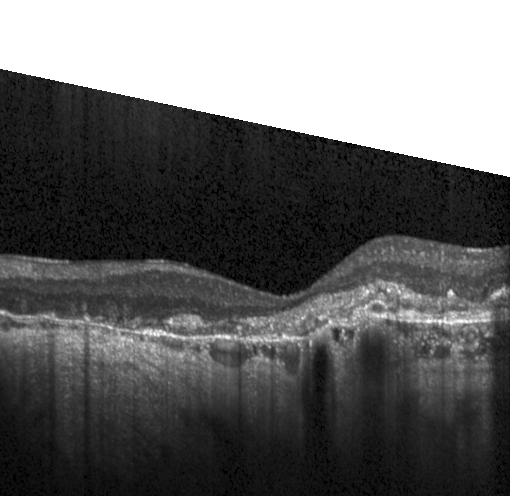

Impression: choroidal neovascularization.